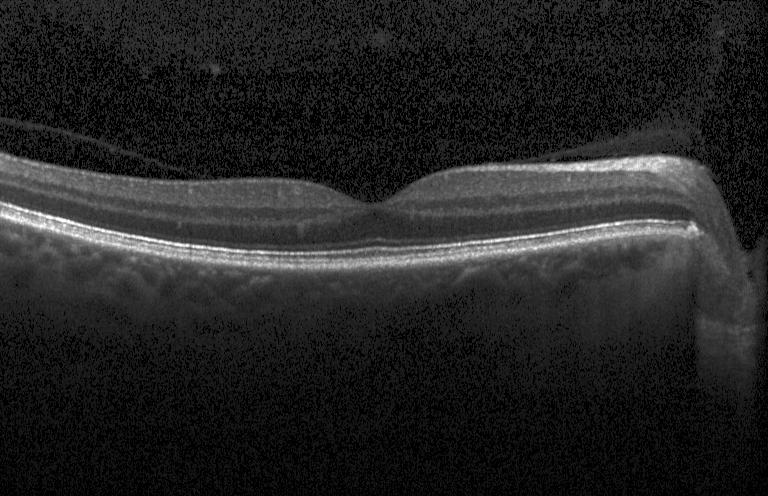 Horizontal scan through the fovea; spectral-domain optical coherence tomography; optical coherence tomography B-scan — Diagnosis: no choroidal neovascularization, diabetic macular edema, or drusen.